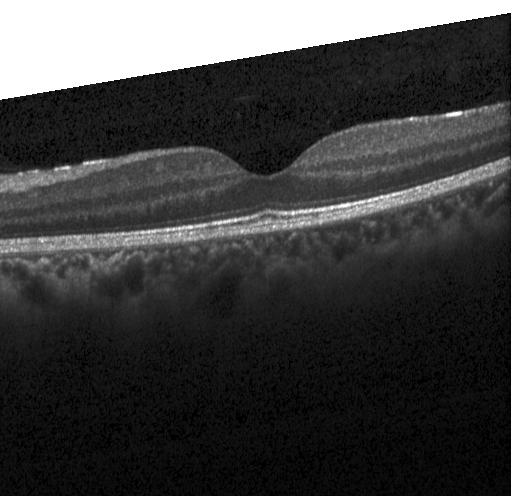

Heidelberg Spectralis OCT system · OCT B-scan · horizontal scan through the fovea · spectral-domain optical coherence tomography — Finding: neither choroidal neovascularization, diabetic macular edema, nor drusen.